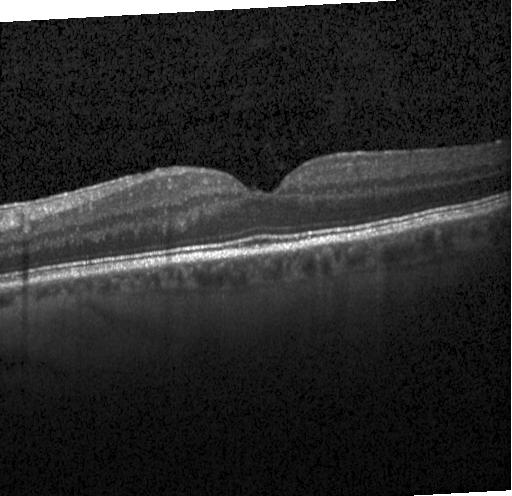
Retinal OCT cross-section
Diagnosis: no evidence of choroidal neovascularization, diabetic macular edema, or drusen.